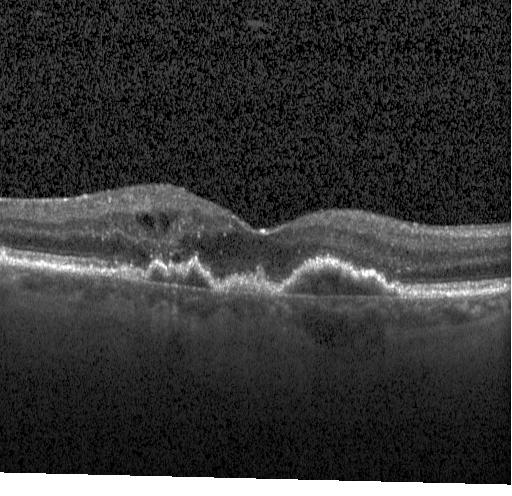
OCT finding: choroidal neovascularization.